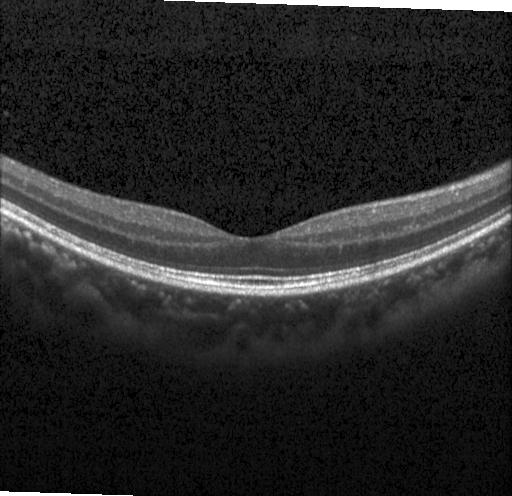

Retinal OCT cross-section, through the macula.
Assessment: no evidence of choroidal neovascularization, diabetic macular edema, or drusen.